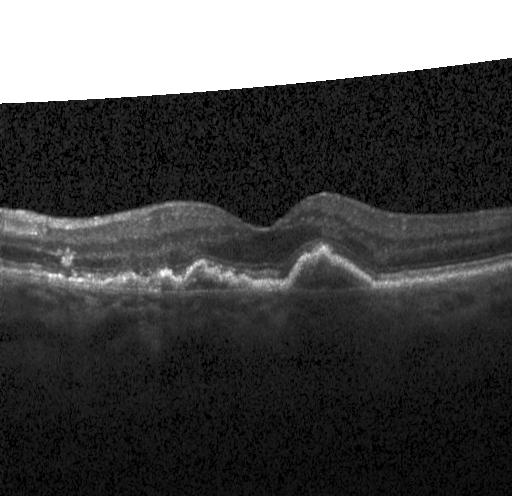

This B-scan demonstrates choroidal neovascularization (CNV).